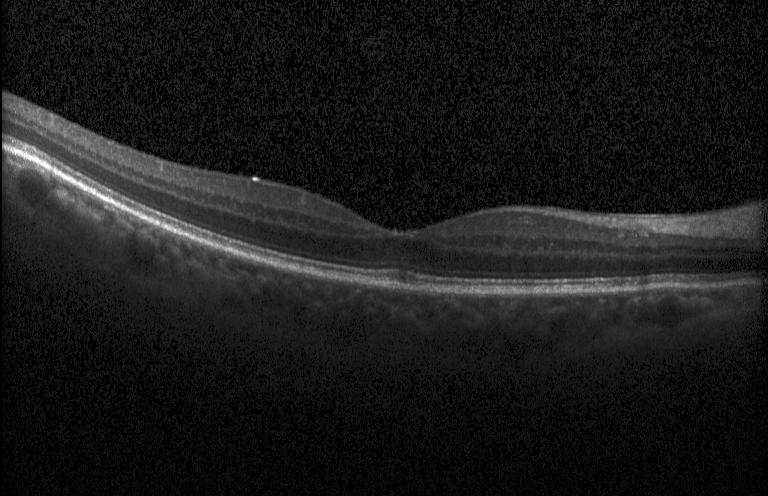
Diagnosis: no choroidal neovascularization, diabetic macular edema, or drusen.